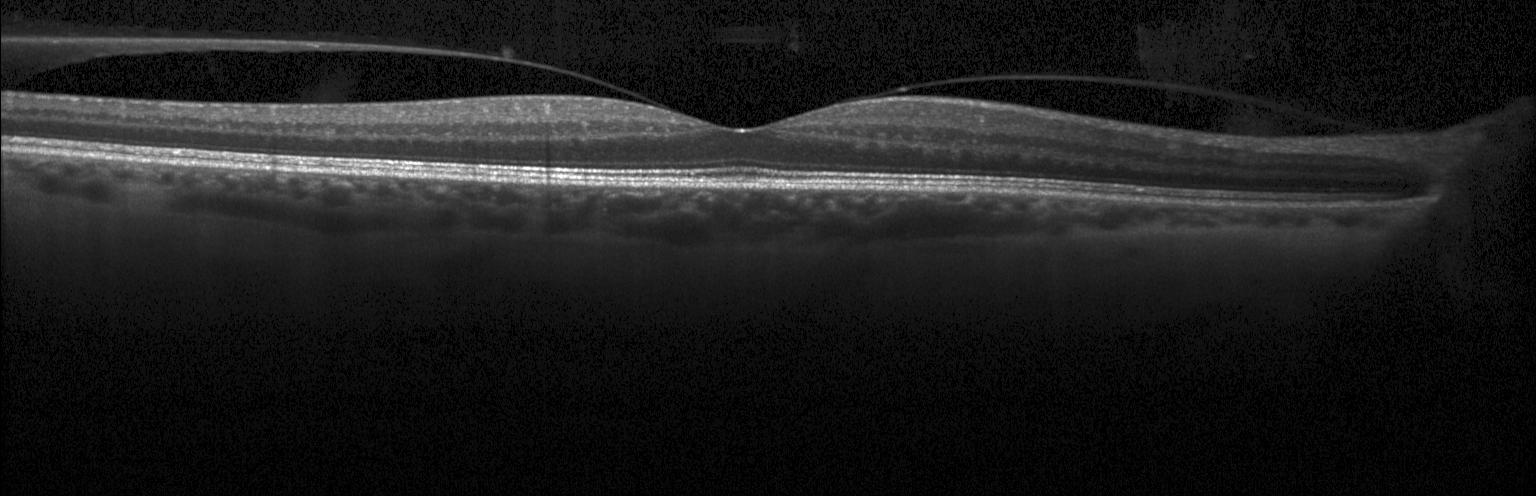
Optical coherence tomography scan. Spectral-domain OCT. Heidelberg Spectralis OCT system. Through the macula. Finding: no choroidal neovascularization, diabetic macular edema, or drusen.